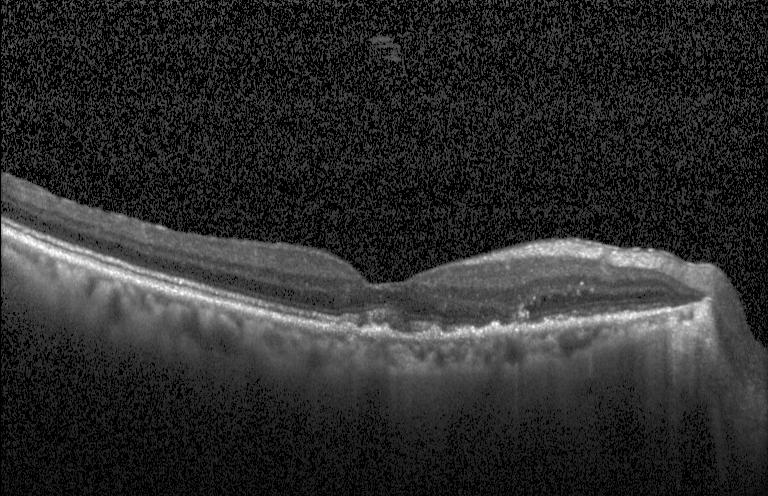

OCT line scan, SD-OCT, Heidelberg Spectralis.
Impression: CNV.